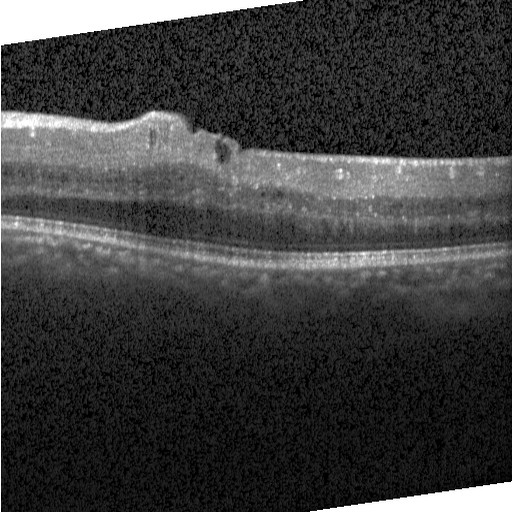 Acquired on a Heidelberg Spectralis · optical coherence tomography B-scan
Dx: diabetic macular edema.